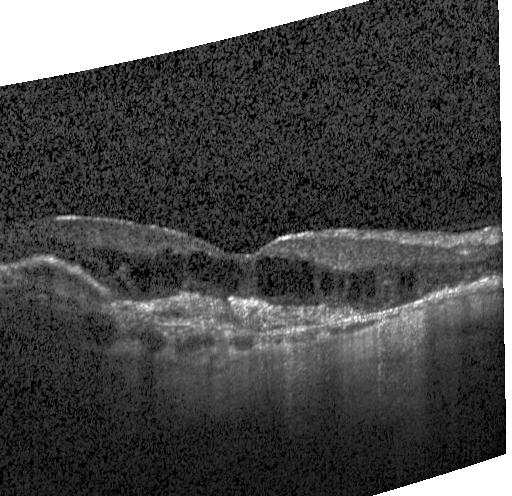
Instrument: Heidelberg Spectralis, OCT B-scan.
Finding: a choroidal neovascular membrane.